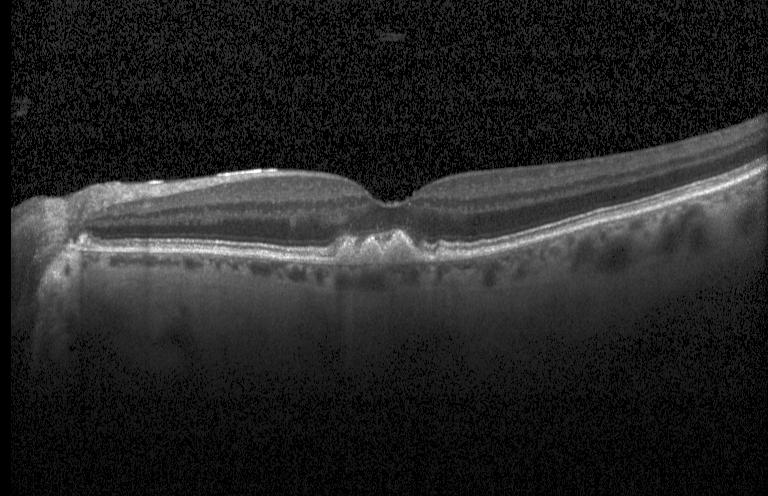
OCT B-scan. Heidelberg Spectralis. Spectral-domain optical coherence tomography.
Impression: drusen.